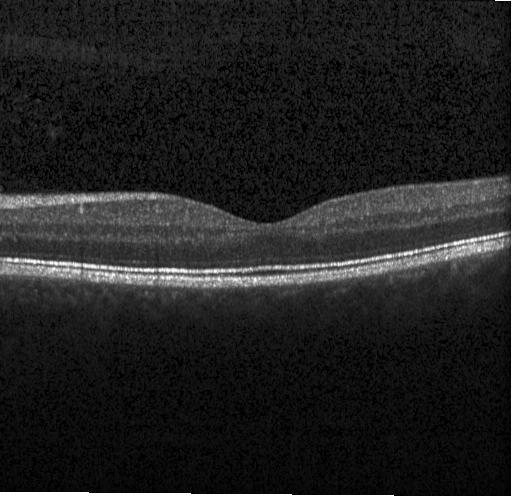 SD-OCT. Acquired on a Heidelberg Spectralis. Retinal OCT B-scan.
This B-scan demonstrates no CNV, DME, or drusen.